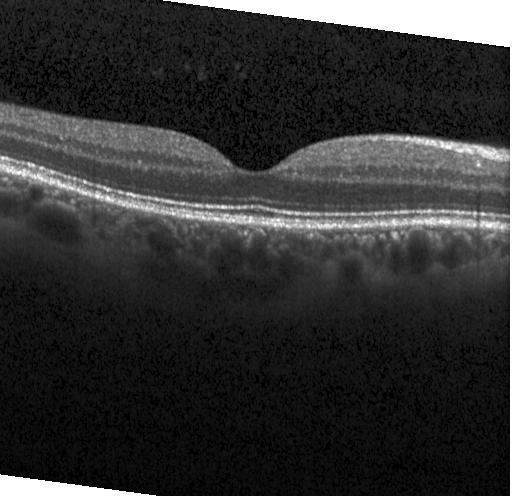
Fovea-centered; SD-OCT; optical coherence tomography scan; instrument: Heidelberg Spectralis. Assessment: no choroidal neovascularization, diabetic macular edema, or drusen.